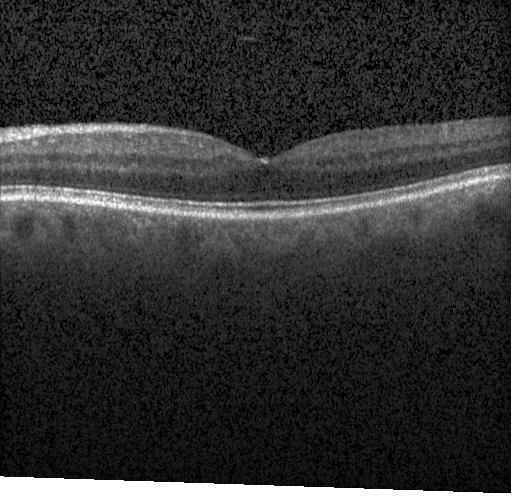

Centered on the fovea · retinal OCT B-scan · spectral-domain OCT · instrument: Heidelberg Spectralis
Dx: no choroidal neovascularization, diabetic macular edema, or drusen.